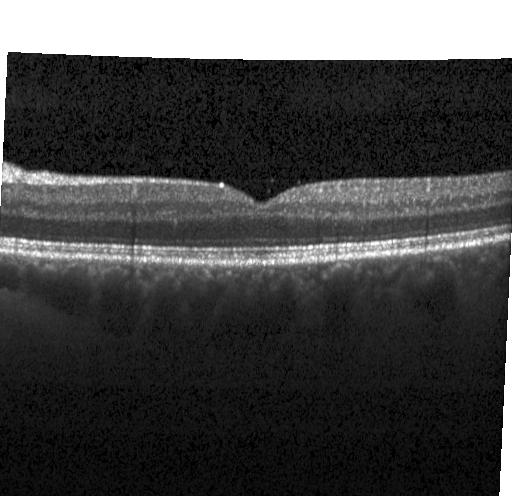
Heidelberg Spectralis OCT system, OCT line scan, spectral-domain optical coherence tomography, macular scan — Dx: no choroidal neovascularization, no diabetic macular edema, and no drusen.